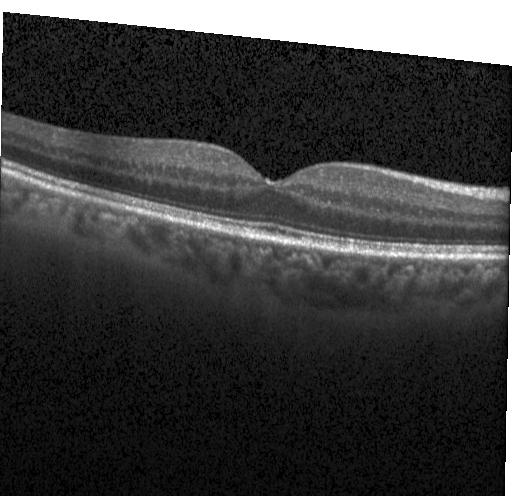
Retinal OCT B-scan; spectral-domain OCT; Heidelberg Spectralis; horizontal scan through the fovea — The scan shows neither choroidal neovascularization, diabetic macular edema, nor drusen.